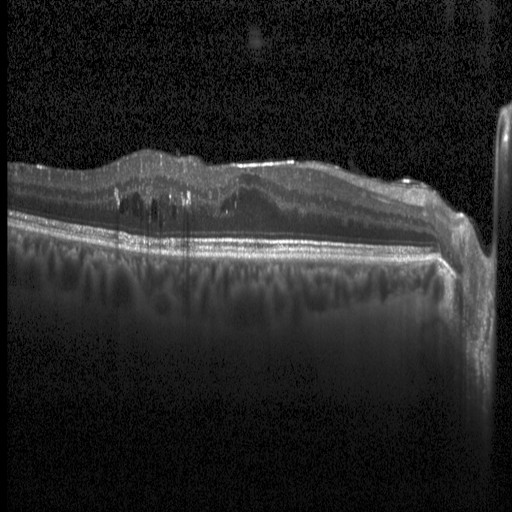
Finding: diabetic macular edema (DME).